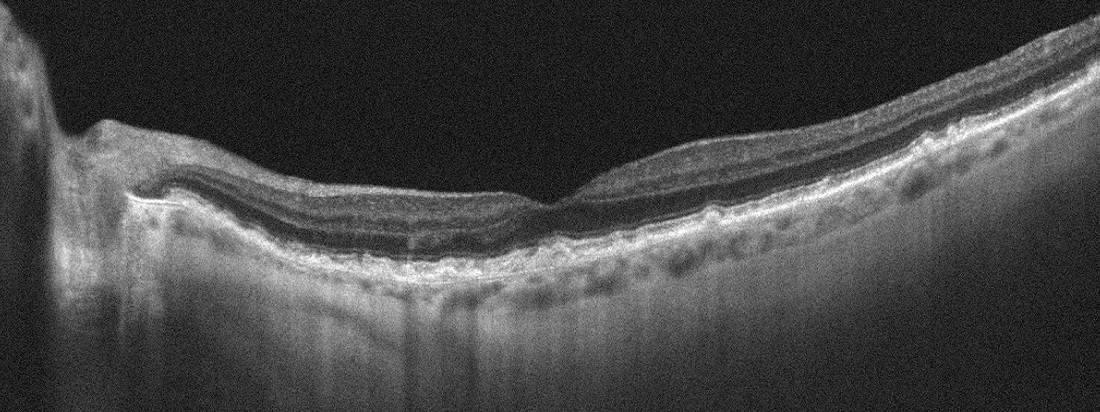

Diagnosis: AMD.